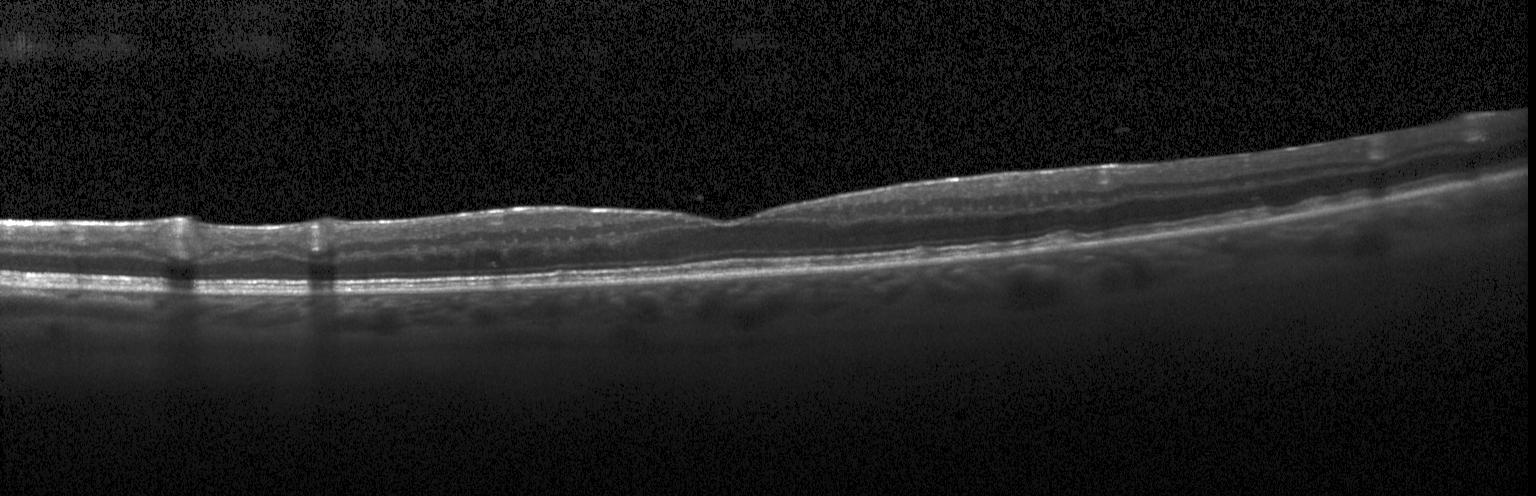 Finding: no choroidal neovascularization, diabetic macular edema, or drusen.